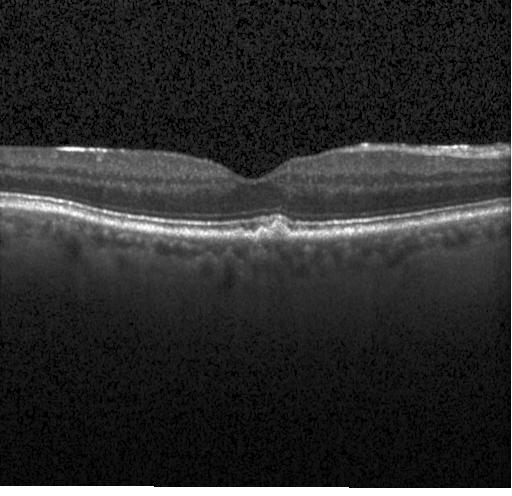
Diagnosis: sub-RPE drusenoid deposits.